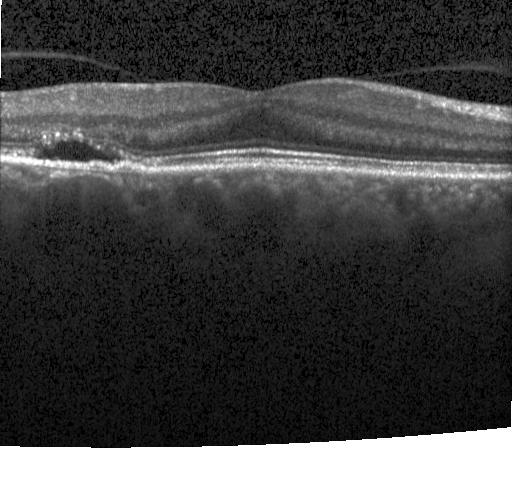 Retinal OCT cross-section. CNV.